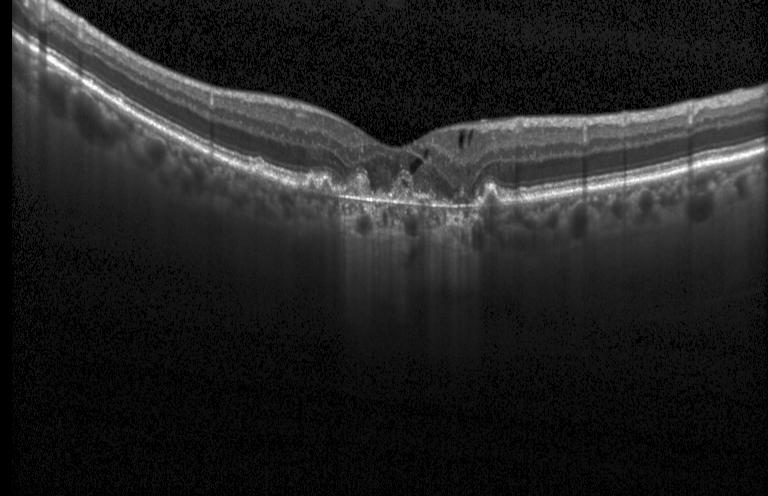 Heidelberg Spectralis OCT system. OCT line scan. Spectral-domain optical coherence tomography — Impression: choroidal neovascularization.